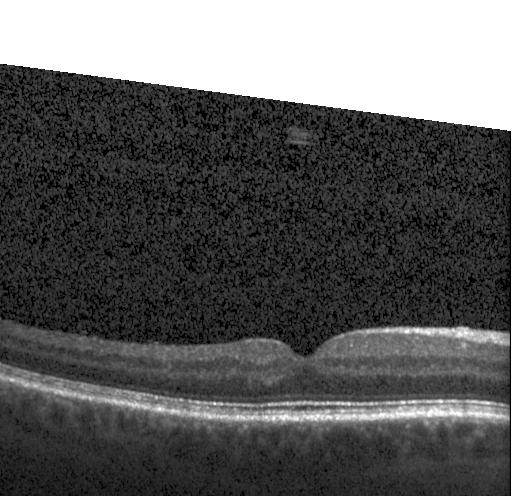

OCT B-scan — Finding: no choroidal neovascularization, diabetic macular edema, or drusen.